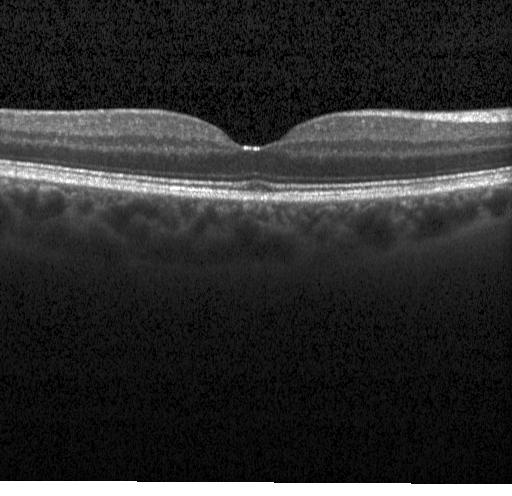
Spectral-domain OCT B-scan: no CNV, no DME, and no drusen.